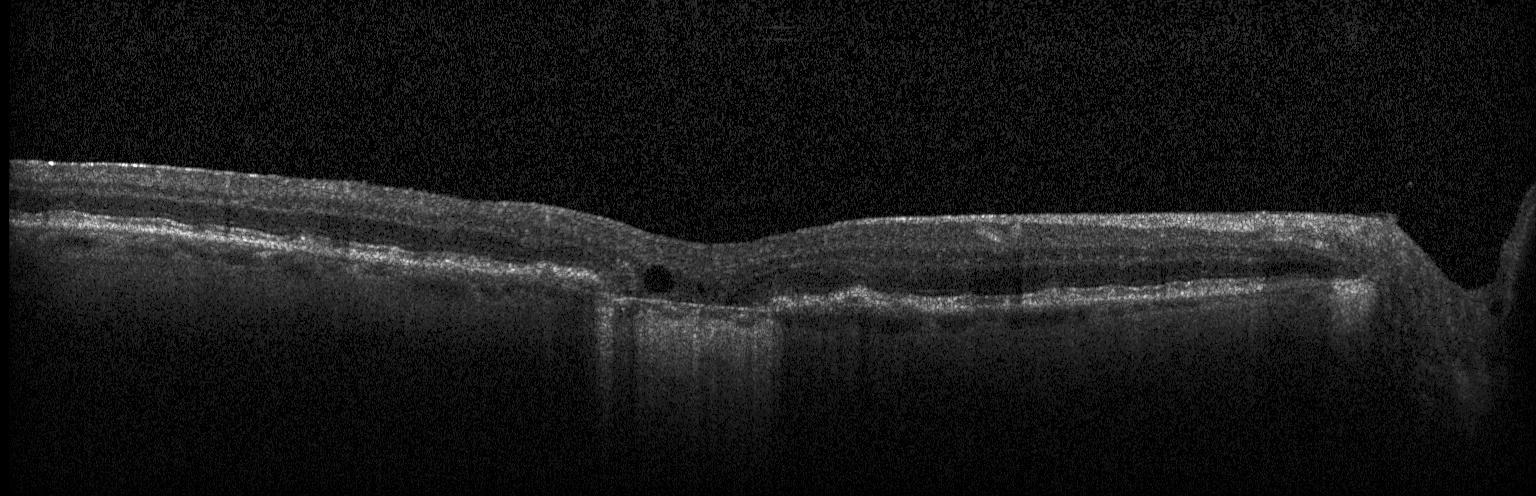

Through the macula. SD-OCT. OCT line scan. Heidelberg Spectralis OCT system — OCT finding: a choroidal neovascular membrane.